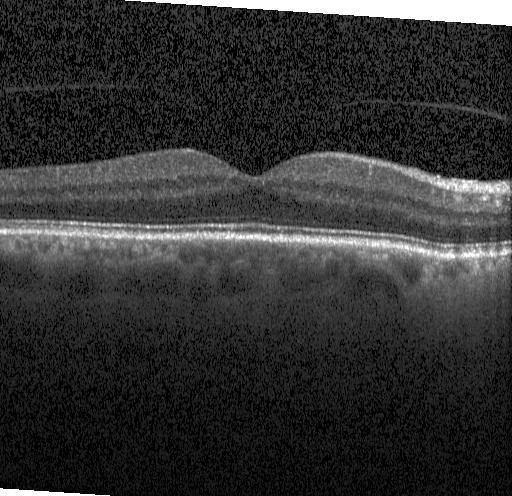
Retinal OCT cross-section showing no choroidal neovascularization, no diabetic macular edema, and no drusen.